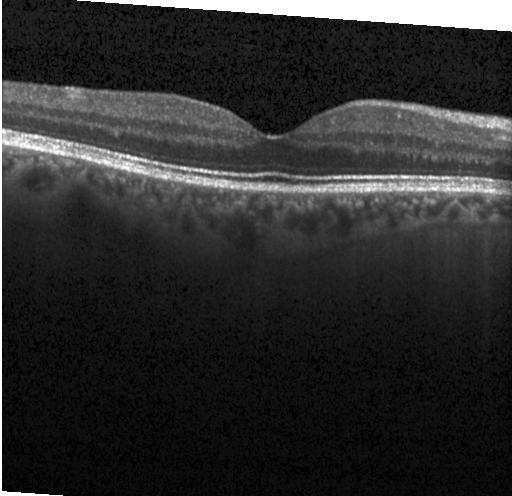 Spectral-domain OCT · optical coherence tomography B-scan. OCT finding: neither CNV, DME, nor drusen.